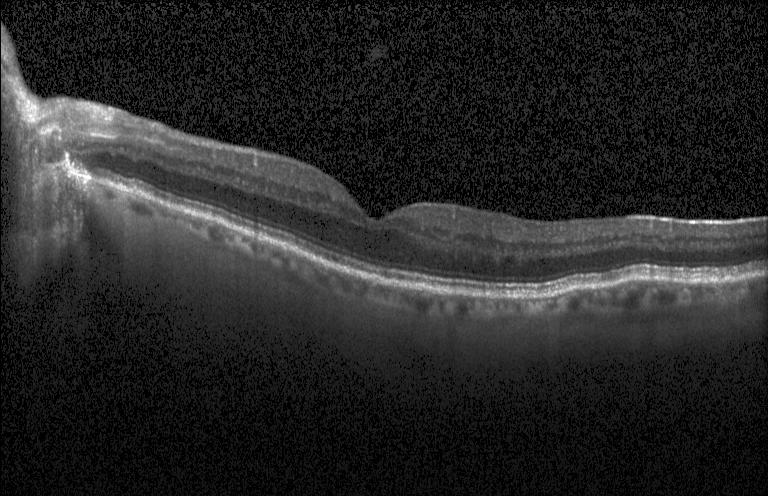

Retinal OCT cross-section.
This B-scan demonstrates neither choroidal neovascularization, diabetic macular edema, nor drusen.